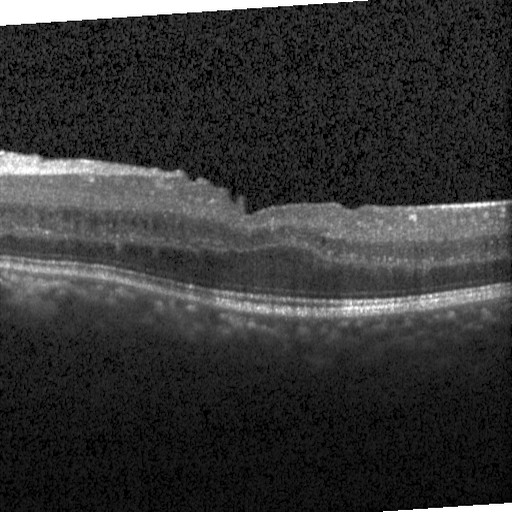

Retinal OCT cross-section
Macular OCT: diabetic macular edema (DME).